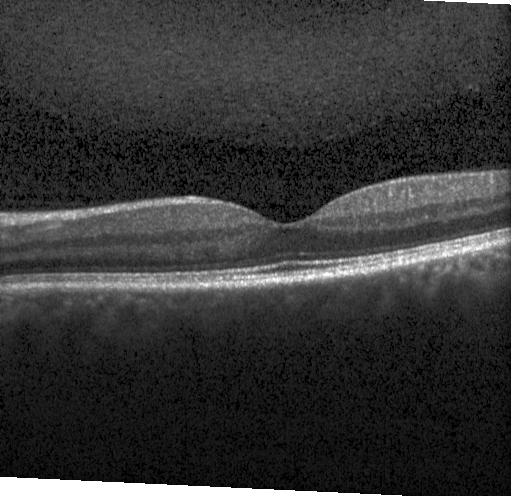
Diagnosis: no CNV, no DME, and no drusen.